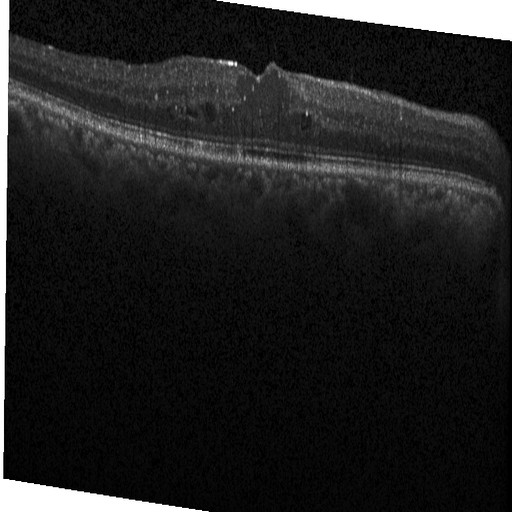

Assessment: diabetic macular edema.